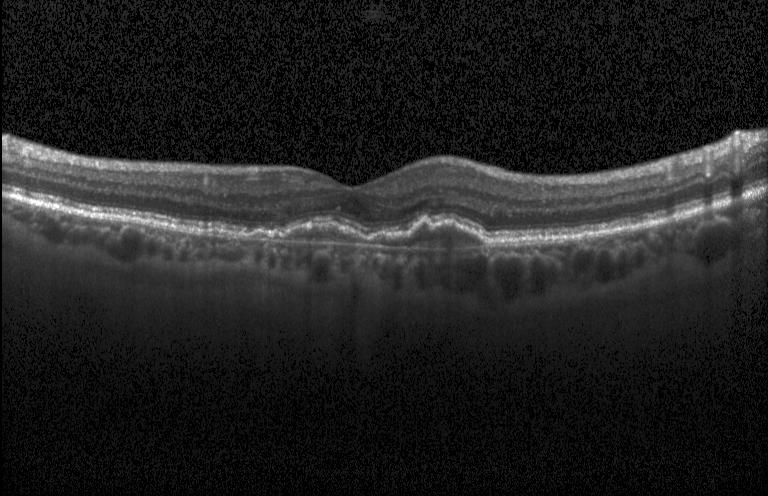 Optical coherence tomography scan.
Assessment: choroidal neovascularization.